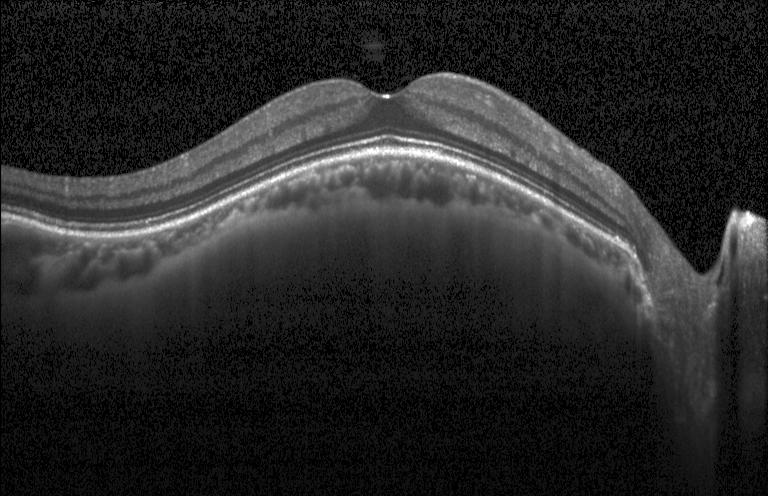 The scan shows no choroidal neovascularization, no diabetic macular edema, and no drusen.